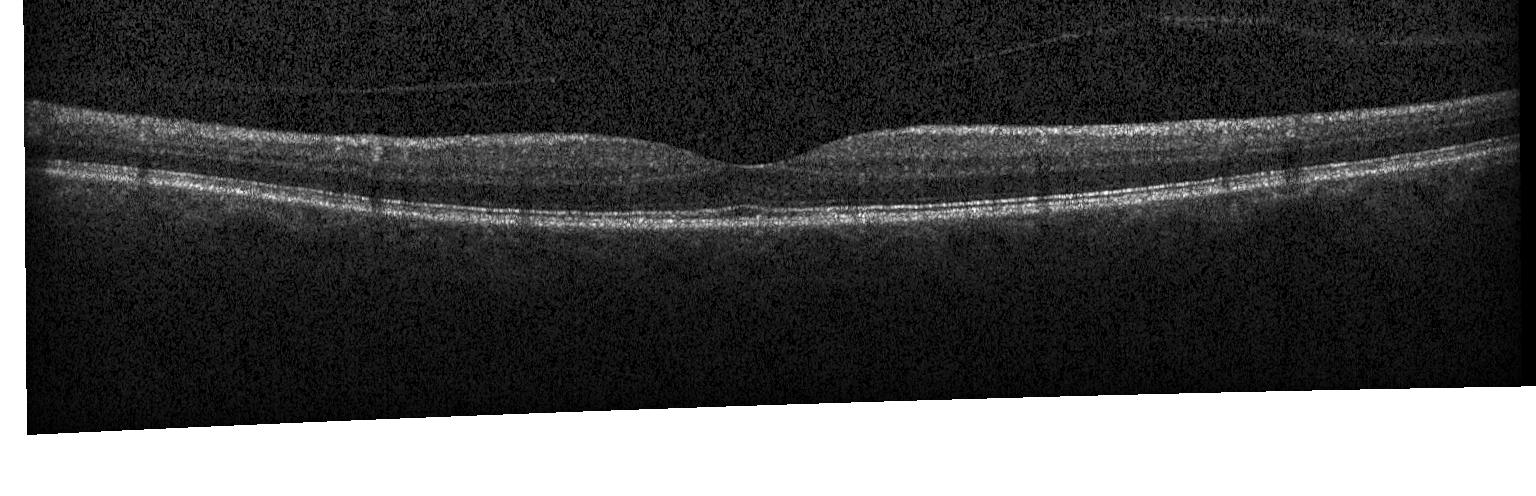
Optical coherence tomography B-scan. Finding: no evidence of CNV, DME, or drusen.